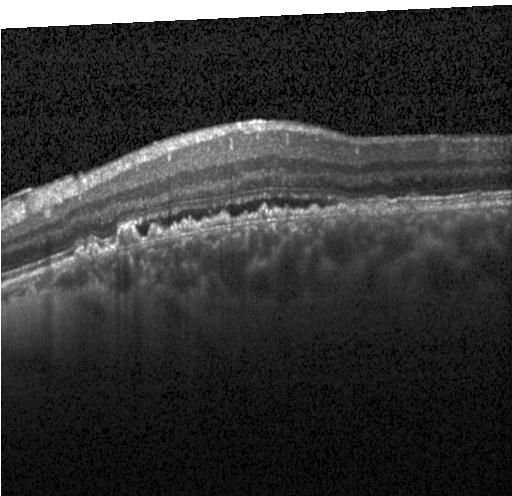 Macular OCT demonstrating a choroidal neovascular membrane.